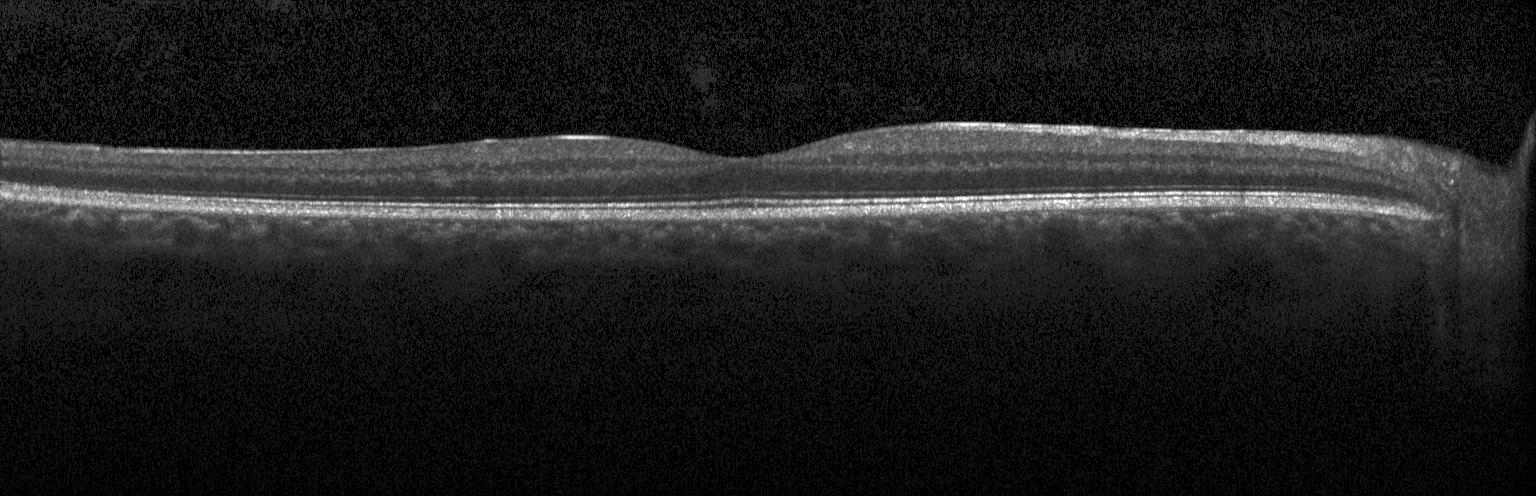 Instrument: Heidelberg Spectralis. Macular scan. Optical coherence tomography B-scan. Spectral-domain OCT.
Diagnosis: neither CNV, DME, nor drusen.